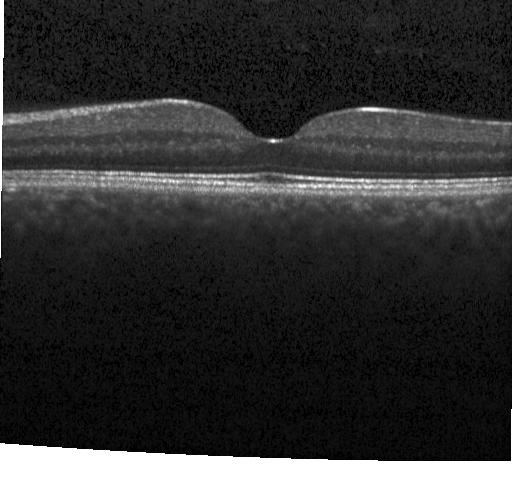

The scan shows no choroidal neovascularization, no diabetic macular edema, and no drusen.